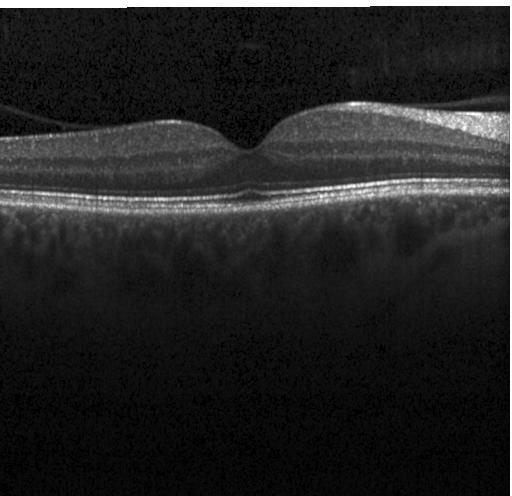

Spectral-domain optical coherence tomography. OCT line scan. Heidelberg Spectralis. This B-scan demonstrates neither choroidal neovascularization, diabetic macular edema, nor drusen.